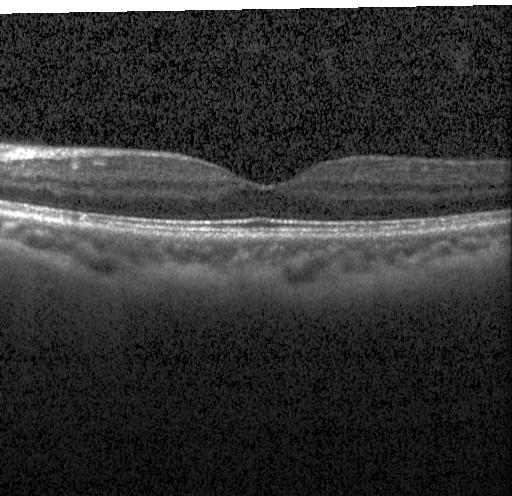 Finding: neither CNV, DME, nor drusen.